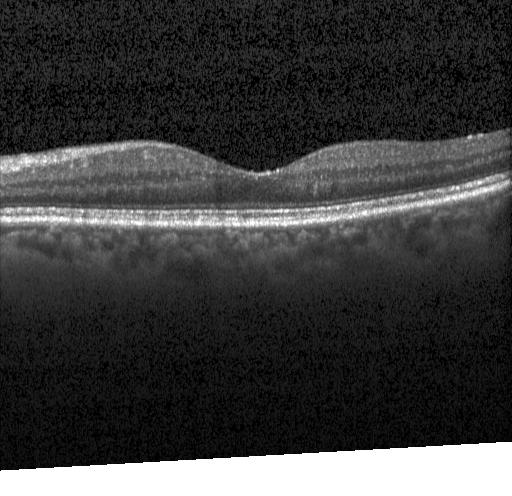

No choroidal neovascularization, no diabetic macular edema, and no drusen.